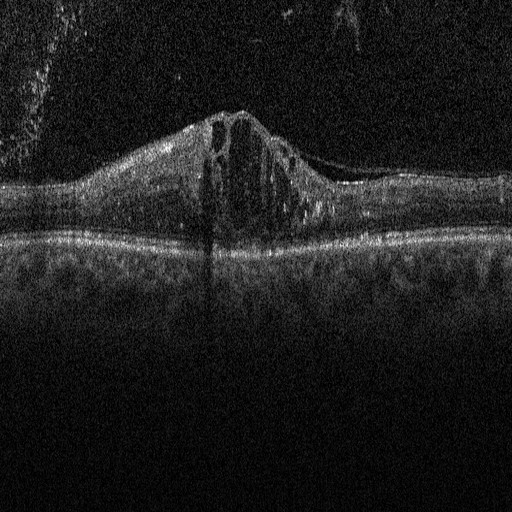

Retinal OCT B-scan; fovea-centered; instrument: Heidelberg Spectralis
Finding: diabetic macular edema.